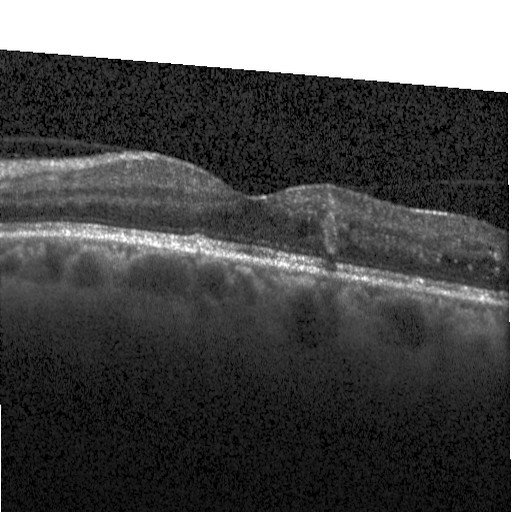
Through the macula. SD-OCT. Optical coherence tomography scan.
Diagnosis: diabetic macular edema.